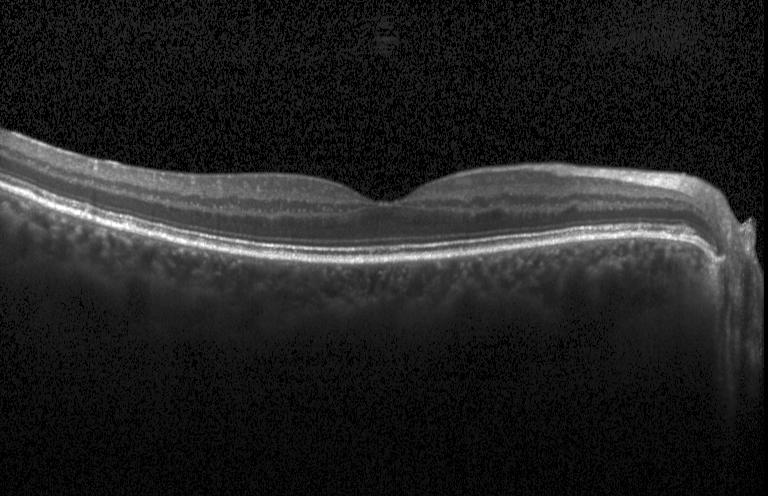

Assessment: no evidence of choroidal neovascularization, diabetic macular edema, or drusen.